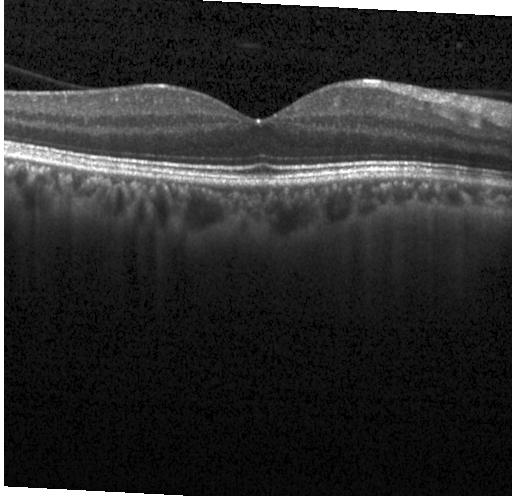

Instrument: Heidelberg Spectralis; centered on the fovea; OCT line scan; spectral-domain OCT. This B-scan demonstrates neither CNV, DME, nor drusen.